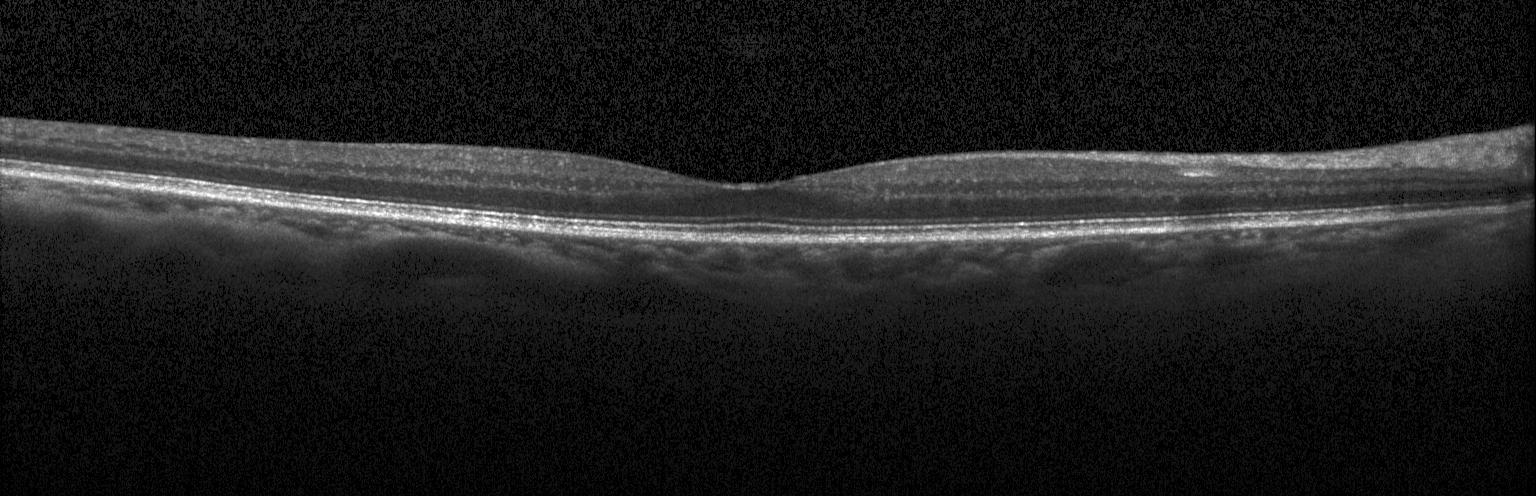

Retinal OCT cross-section, SD-OCT
This B-scan demonstrates no choroidal neovascularization, diabetic macular edema, or drusen.